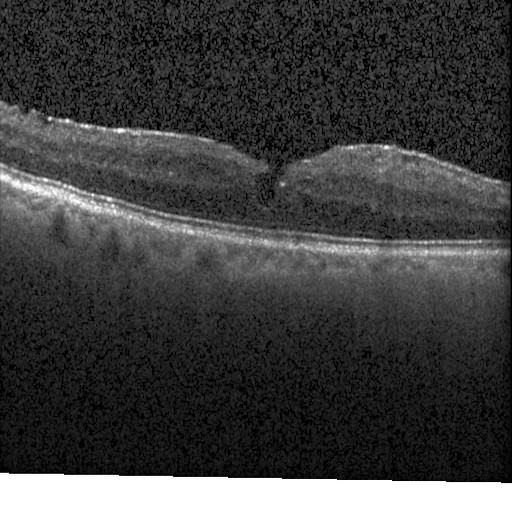

Optical coherence tomography scan, spectral-domain OCT — Diagnosis: DME.